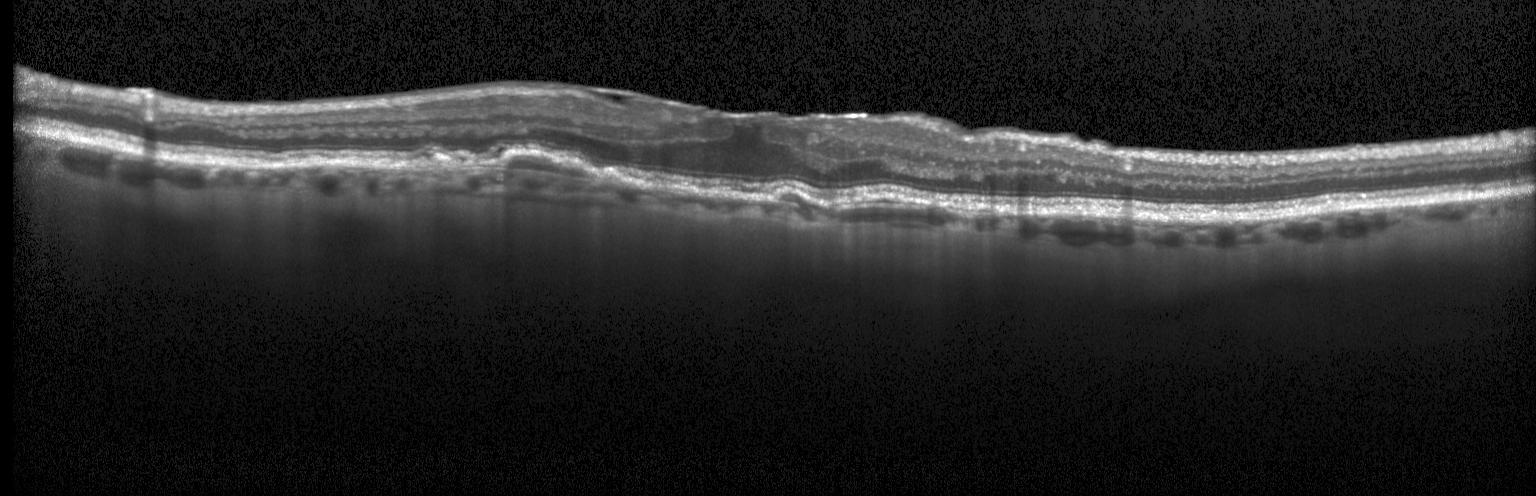
Optical coherence tomography scan
Diagnosis: choroidal neovascularization (CNV).